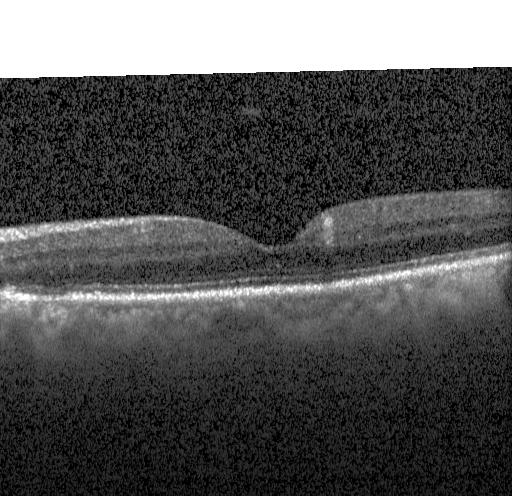 OCT B-scan showing neither choroidal neovascularization, diabetic macular edema, nor drusen.